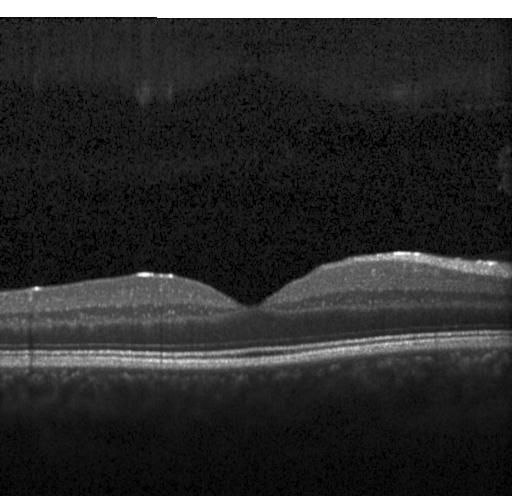

OCT line scan; spectral-domain optical coherence tomography
Assessment: no CNV, DME, or drusen.